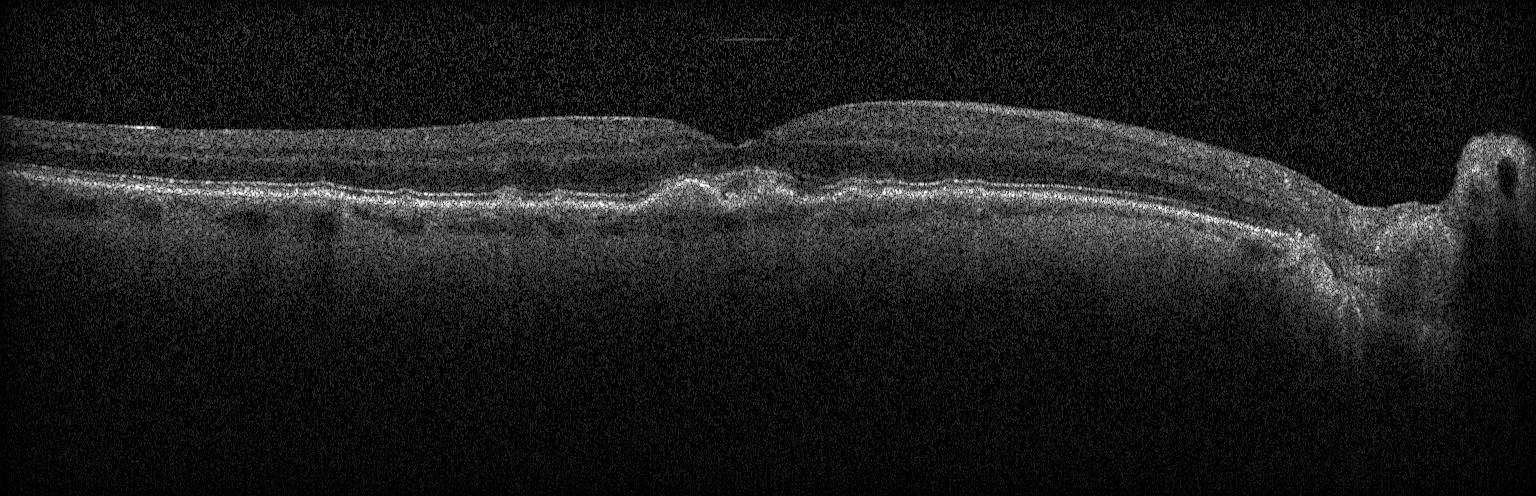
Dx: sub-RPE drusenoid deposits.